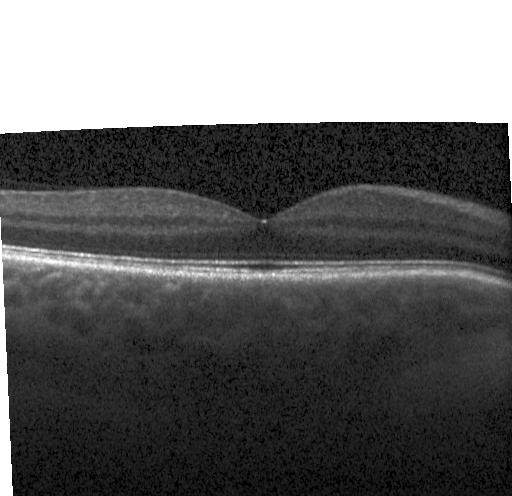 Optical coherence tomography B-scan — Diagnosis: no CNV, no DME, and no drusen.